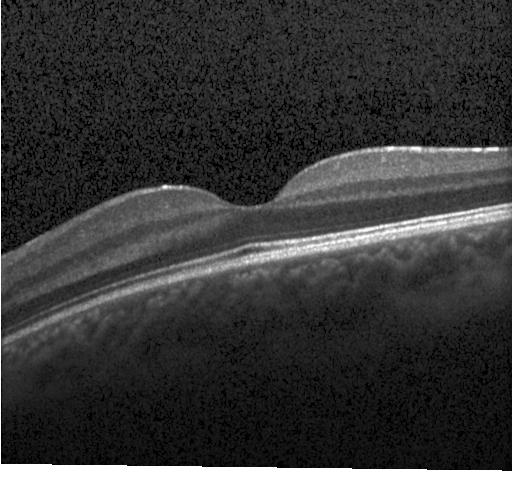
Diagnosis: no choroidal neovascularization, diabetic macular edema, or drusen.